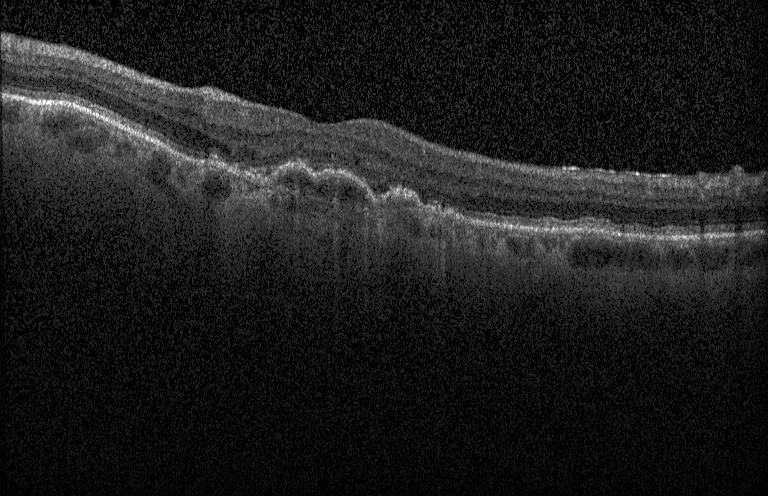
Optical coherence tomography B-scan, acquired on a Heidelberg Spectralis, spectral-domain OCT
OCT finding: choroidal neovascularization (CNV).